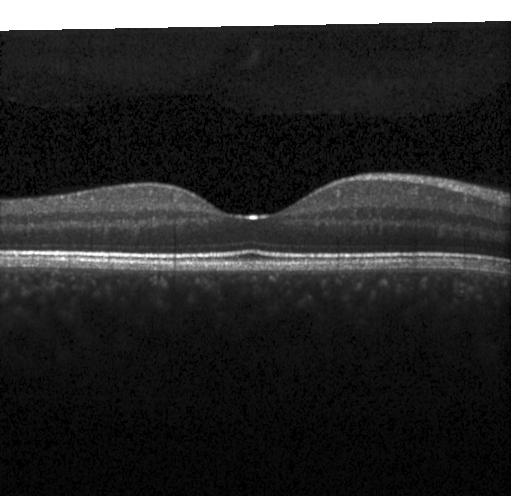
Finding: neither CNV, DME, nor drusen.